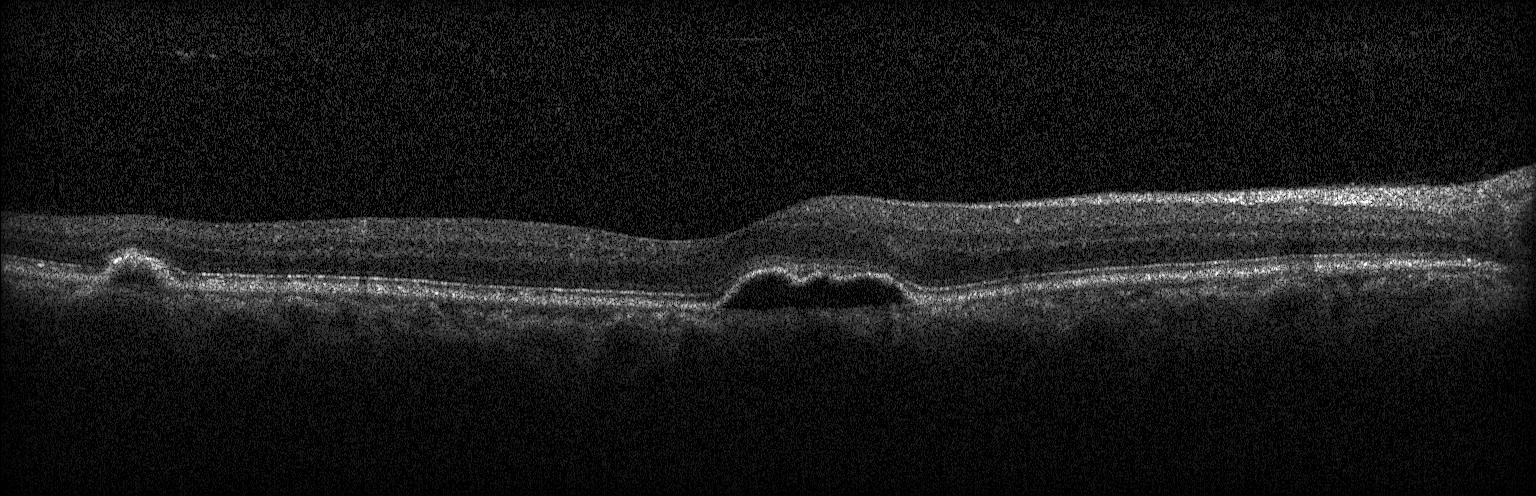

Heidelberg Spectralis OCT system, retinal OCT B-scan
CNV.